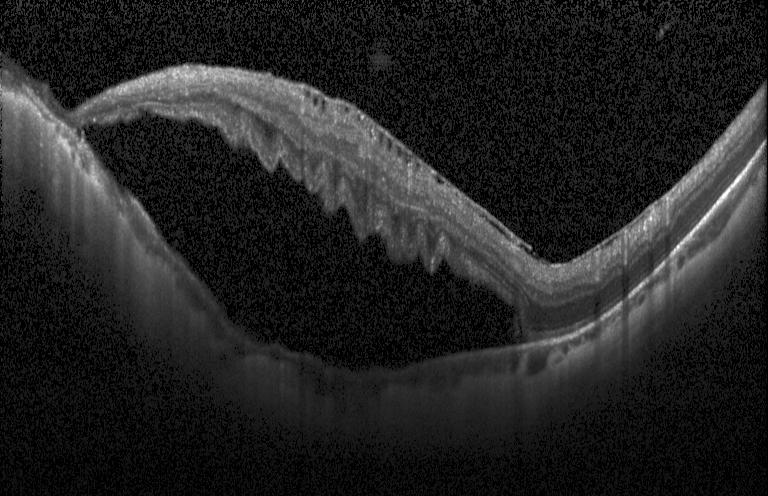
Diagnosis: a choroidal neovascular membrane.